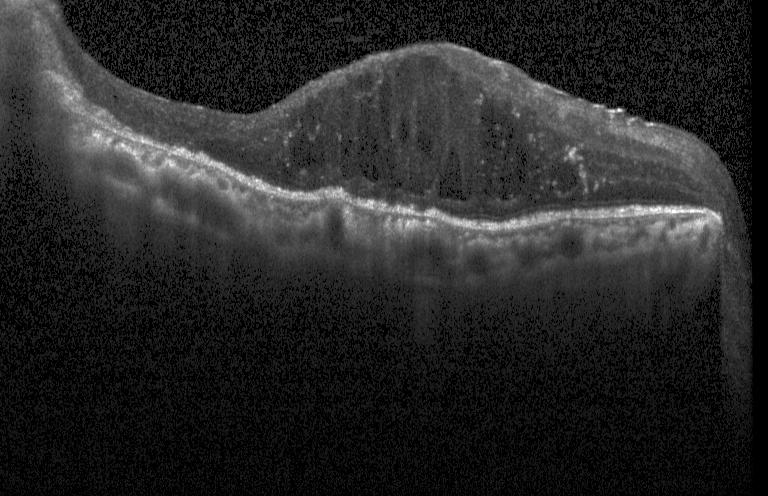

The scan shows diabetic macular edema (DME).